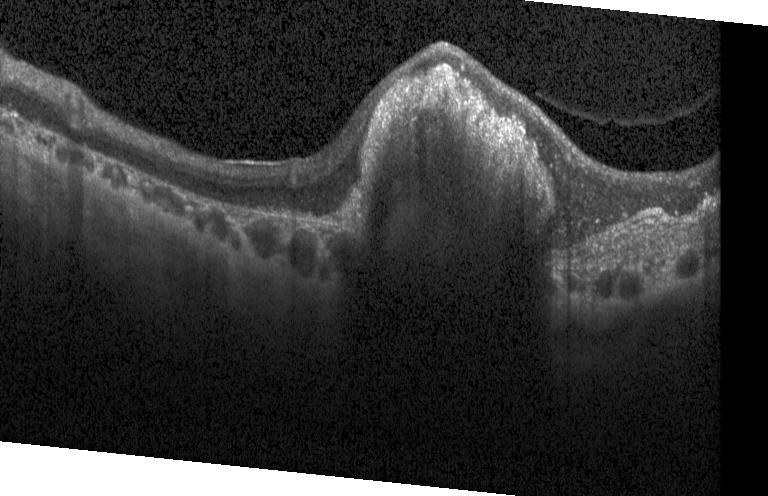
Macular scan · SD-OCT · instrument: Heidelberg Spectralis · OCT B-scan.
Assessment: a choroidal neovascular membrane.